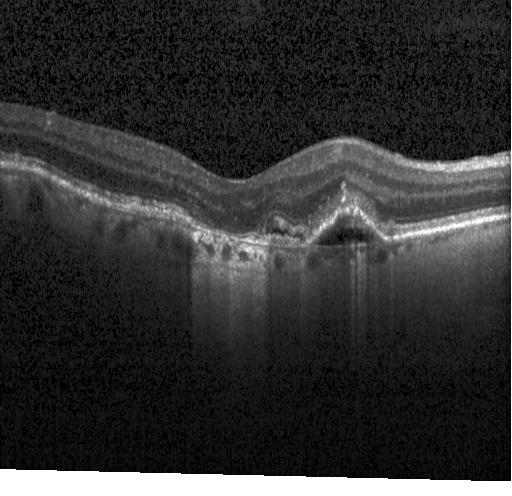

Optical coherence tomography B-scan; acquired on a Heidelberg Spectralis — Impression: choroidal neovascularization (CNV).